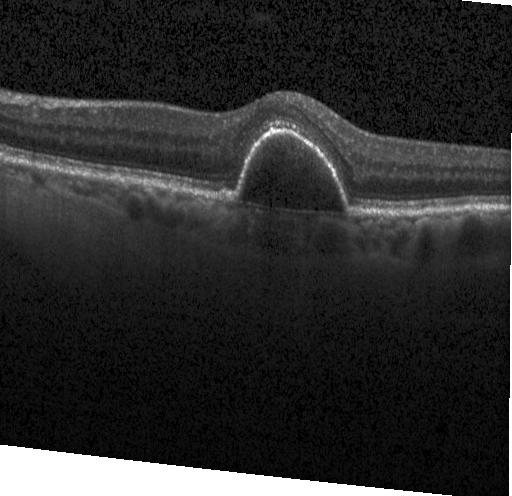

SD-OCT · through the macula · acquired on a Heidelberg Spectralis · retinal OCT B-scan. The scan shows choroidal neovascularization.